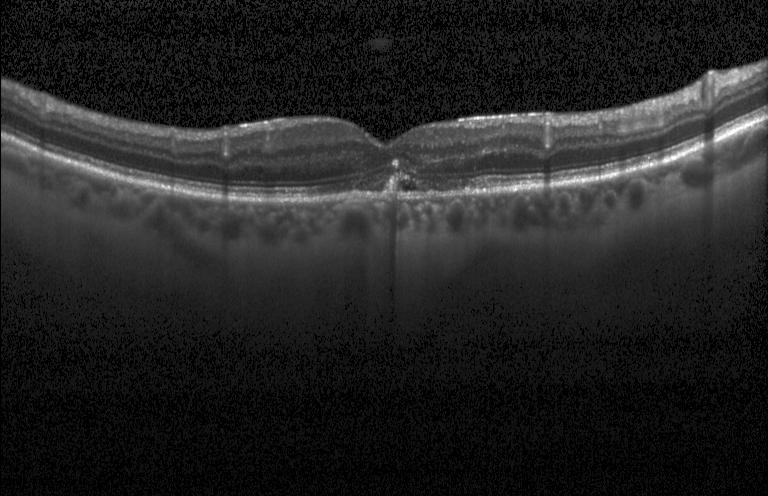
SD-OCT. Optical coherence tomography B-scan — The scan shows a choroidal neovascular membrane.